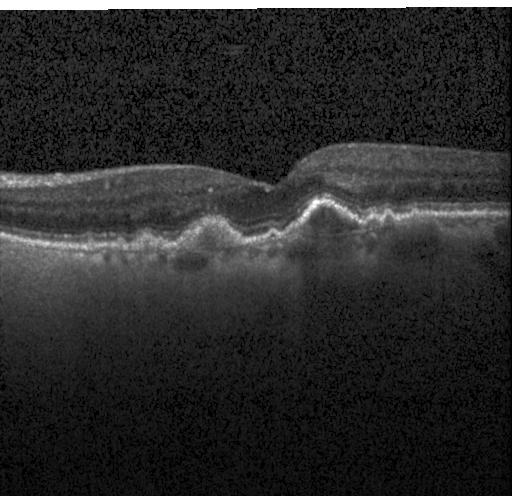

Retinal OCT B-scan; instrument: Heidelberg Spectralis; spectral-domain optical coherence tomography; fovea-centered
The scan shows a choroidal neovascular membrane.